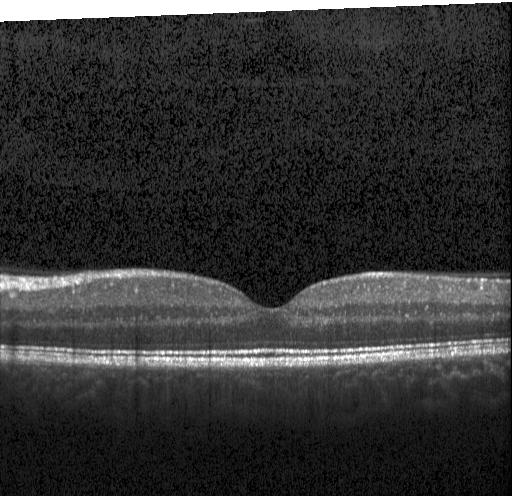
Impression: no choroidal neovascularization, diabetic macular edema, or drusen.